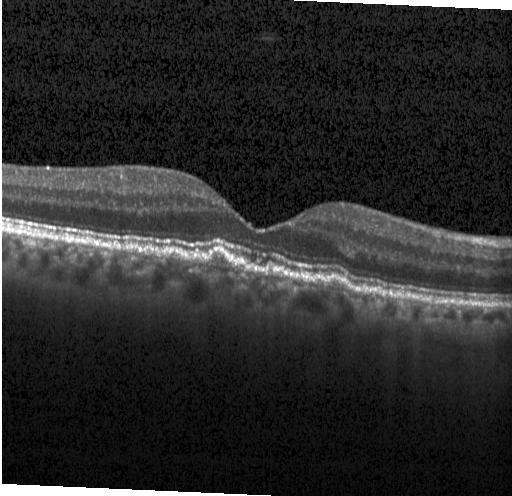 Acquired on a Heidelberg Spectralis; optical coherence tomography B-scan — Diagnosis: drusen.